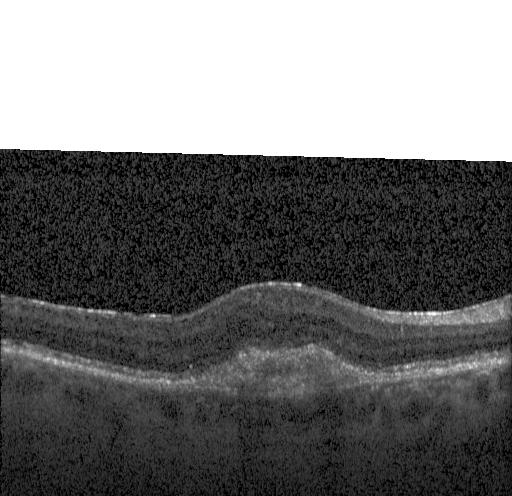 Retinal OCT cross-section. Assessment: choroidal neovascularization.